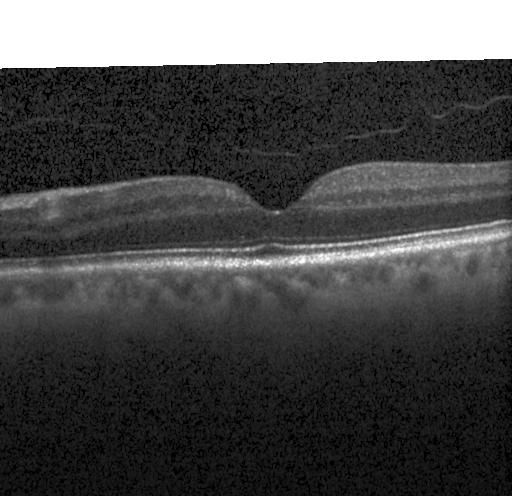
Retinal OCT B-scan. Impression: no CNV, no DME, and no drusen.